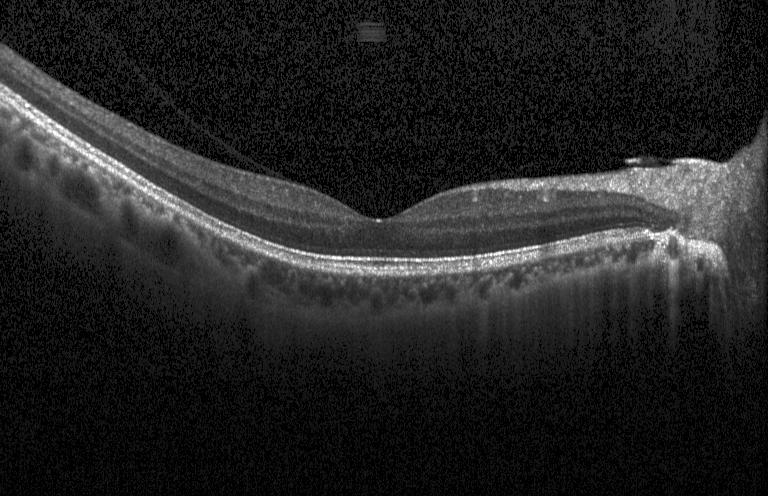

Retinal OCT cross-section.
Assessment: no choroidal neovascularization, diabetic macular edema, or drusen.